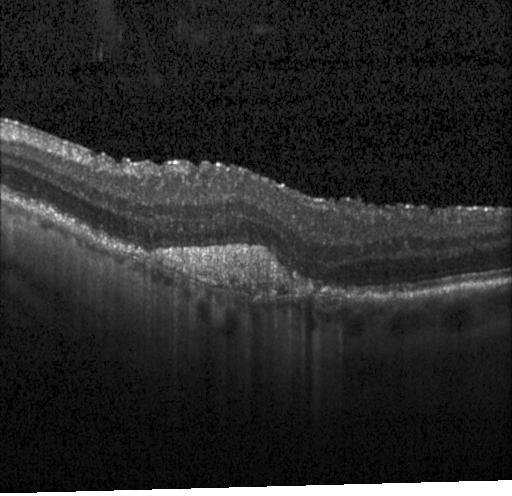

OCT finding: CNV.